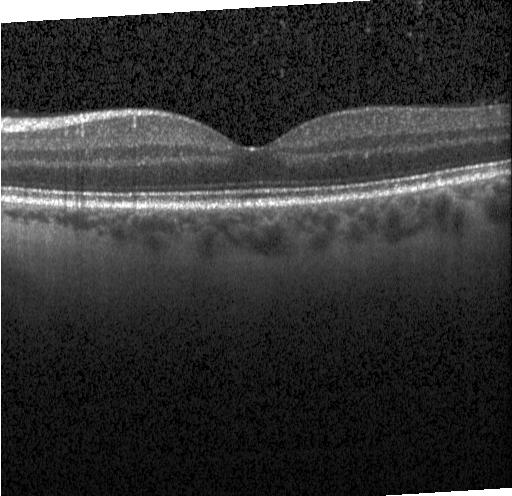
Optical coherence tomography scan — Dx: no evidence of CNV, DME, or drusen.